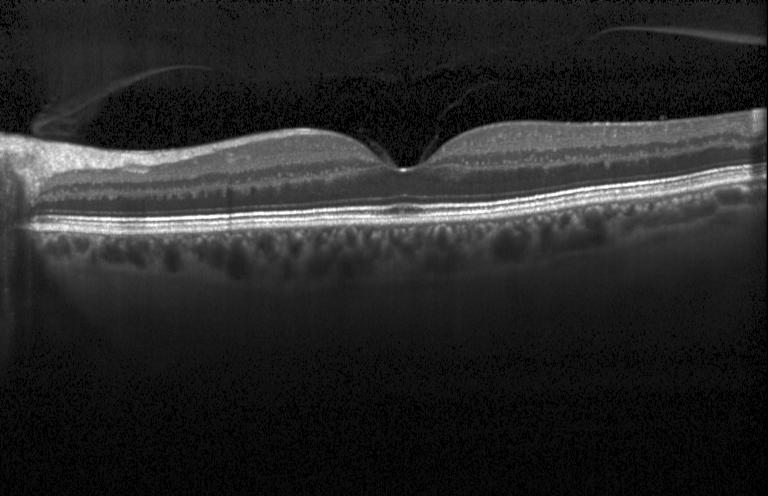

Retinal OCT cross-section showing no choroidal neovascularization, no diabetic macular edema, and no drusen.